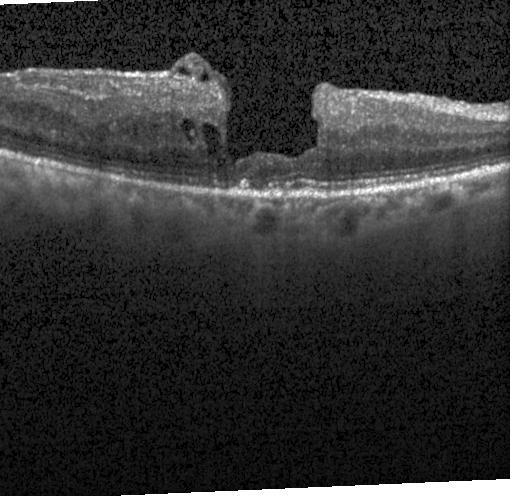
Optical coherence tomography B-scan — Diagnosis: DME.